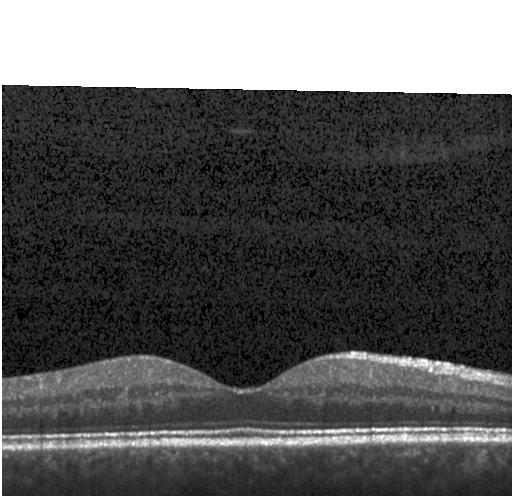 Impression: no evidence of choroidal neovascularization, diabetic macular edema, or drusen.